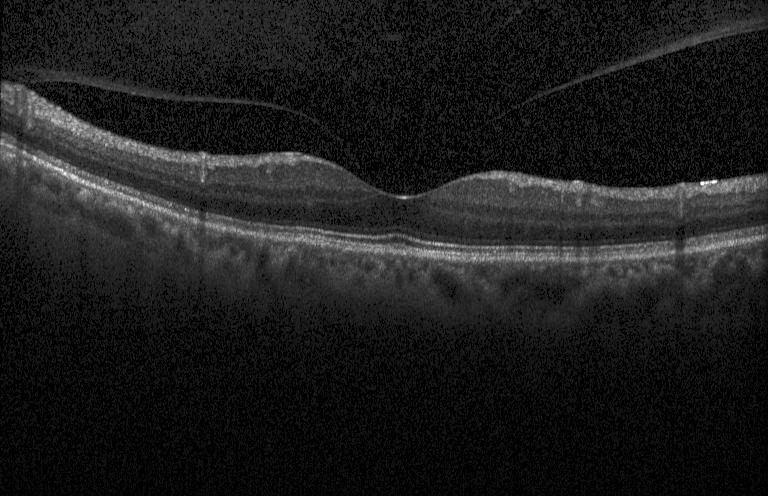

OCT B-scan. Finding: no choroidal neovascularization, no diabetic macular edema, and no drusen.